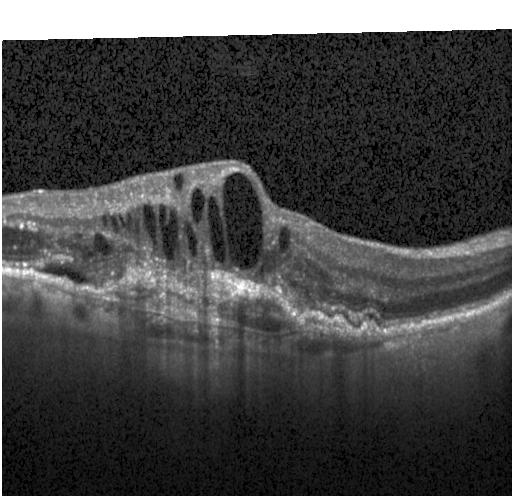

SD-OCT · optical coherence tomography B-scan — Macular OCT: a choroidal neovascular membrane.